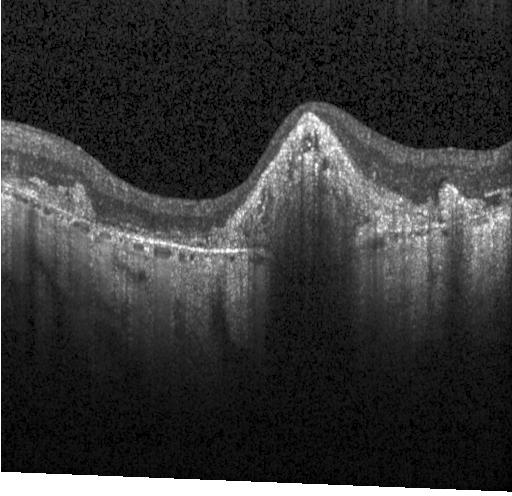

Optical coherence tomography scan.
Finding: a choroidal neovascular membrane.